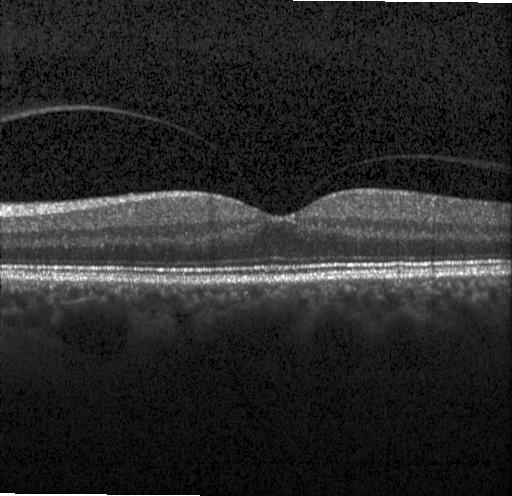 OCT line scan; fovea-centered — Finding: no choroidal neovascularization, diabetic macular edema, or drusen.